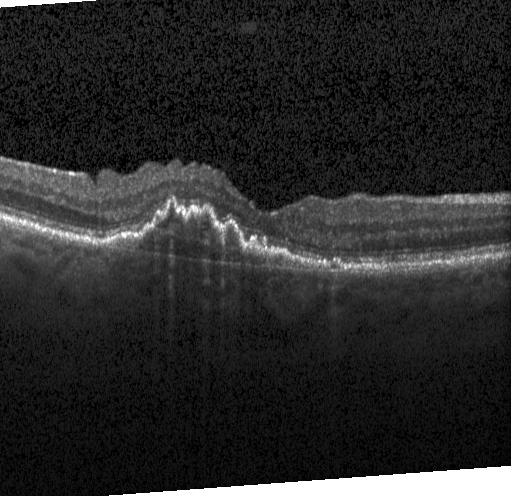

Centered on the fovea. Optical coherence tomography scan. SD-OCT. Instrument: Heidelberg Spectralis.
Impression: choroidal neovascularization.